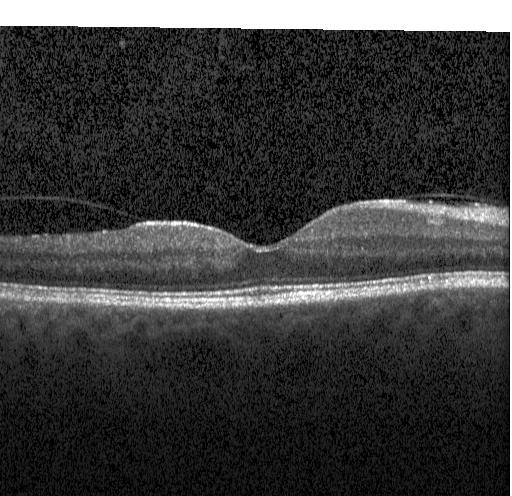 Optical coherence tomography B-scan; Heidelberg Spectralis OCT system; spectral-domain OCT
Diagnosis: neither choroidal neovascularization, diabetic macular edema, nor drusen.